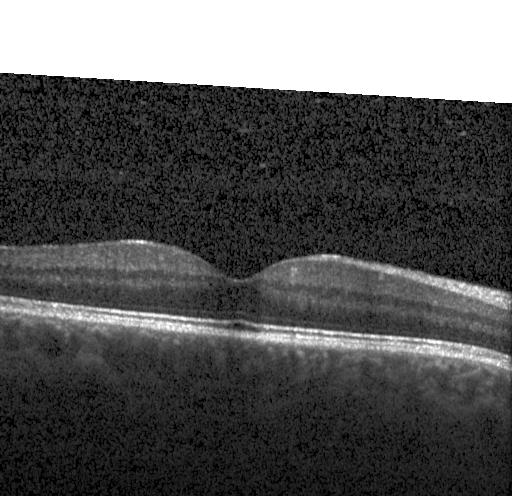
Finding: no evidence of choroidal neovascularization, diabetic macular edema, or drusen.